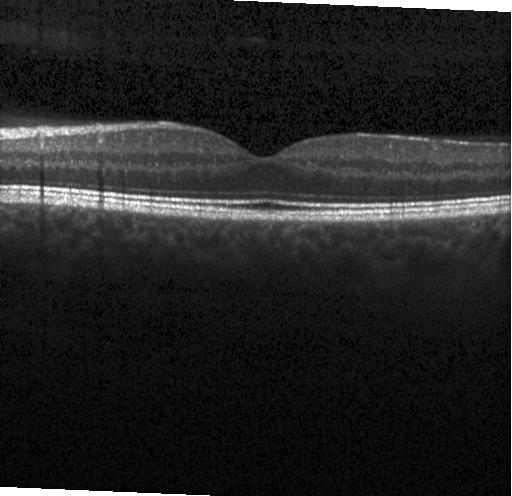
Spectral-domain OCT B-scan: no evidence of choroidal neovascularization, diabetic macular edema, or drusen.